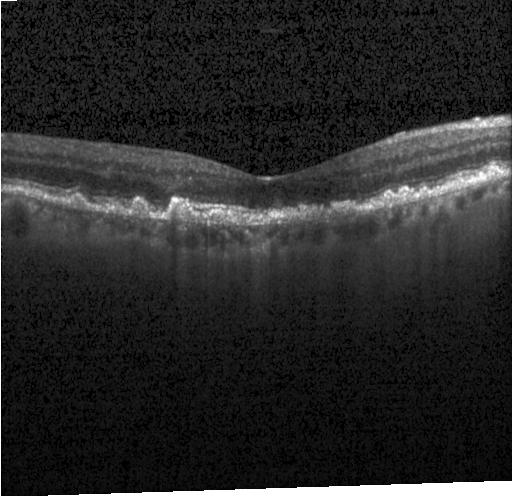 Acquired on a Heidelberg Spectralis, OCT B-scan, spectral-domain OCT — Diagnosis: a choroidal neovascular membrane.